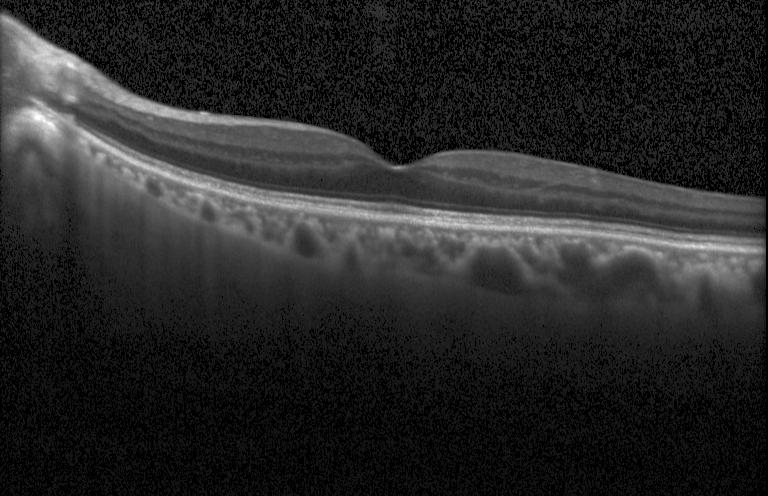

Spectral-domain optical coherence tomography, instrument: Heidelberg Spectralis, OCT line scan. Diagnosis: no evidence of CNV, DME, or drusen.